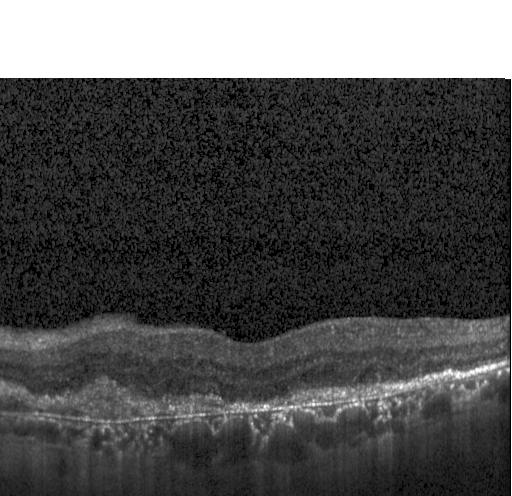 Dx: CNV.